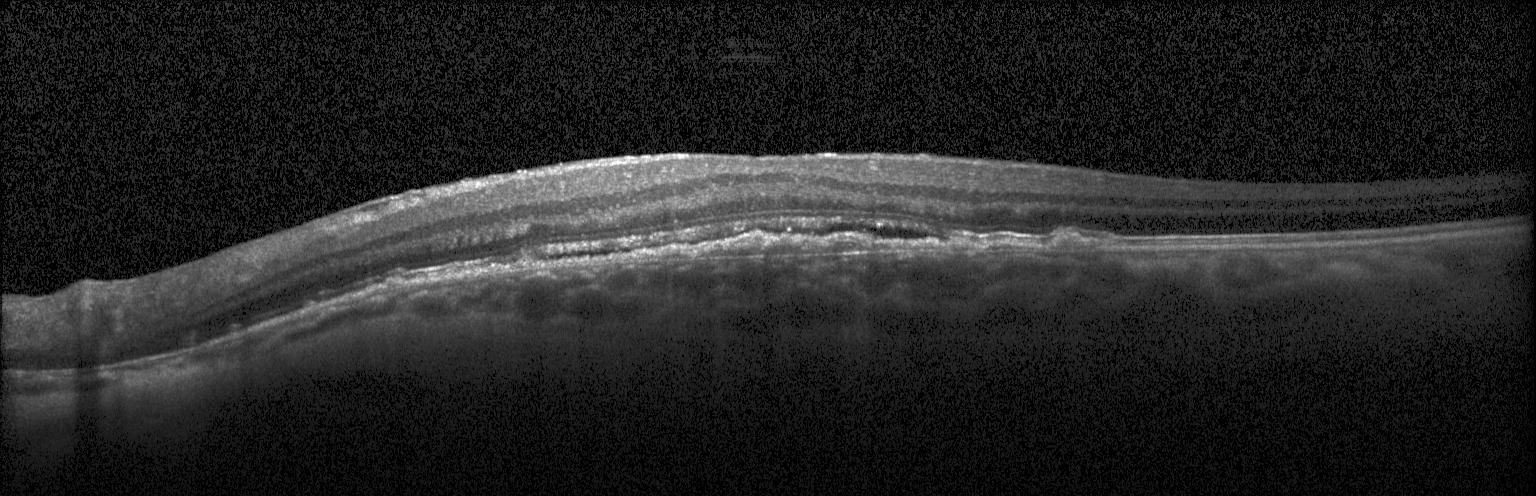

SD-OCT; OCT line scan. Finding: a choroidal neovascular membrane.